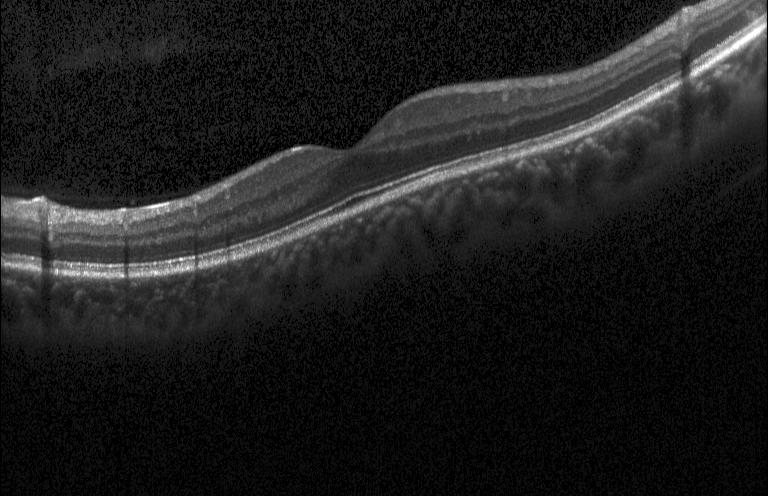

OCT B-scan; Heidelberg Spectralis OCT system
Impression: no CNV, no DME, and no drusen.